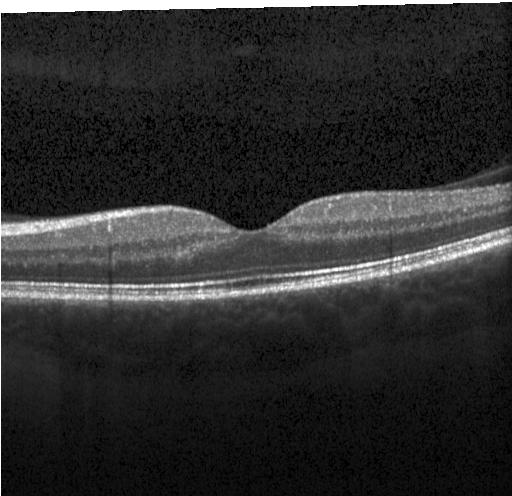
Dx: no choroidal neovascularization, no diabetic macular edema, and no drusen.